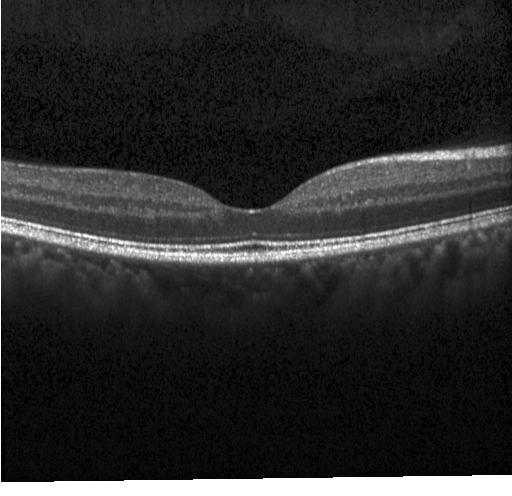 Optical coherence tomography B-scan
Macular OCT: neither choroidal neovascularization, diabetic macular edema, nor drusen.